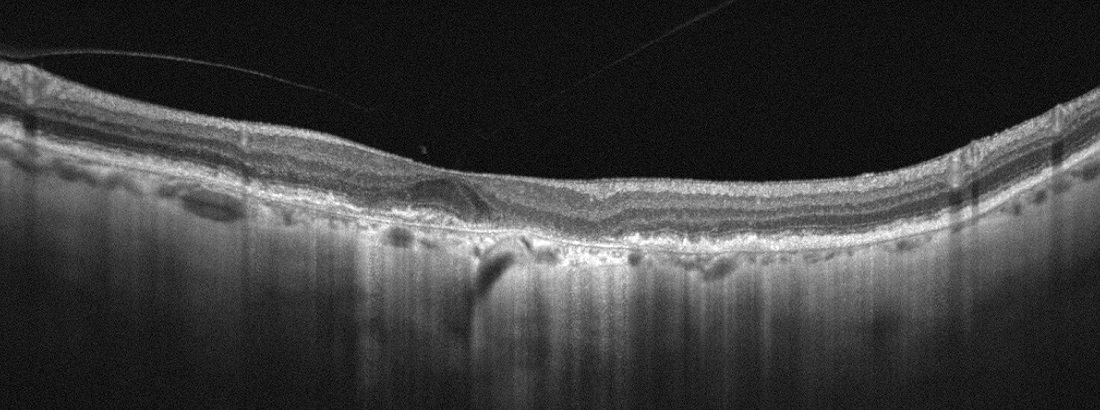

Macular OCT: AMD.